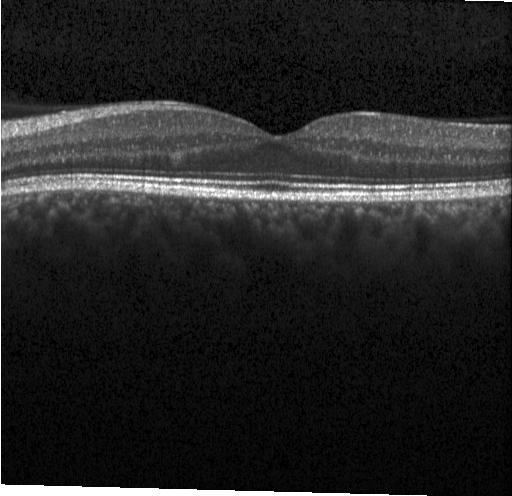

SD-OCT. Macular scan. Heidelberg Spectralis. Optical coherence tomography B-scan
Diagnosis: neither CNV, DME, nor drusen.